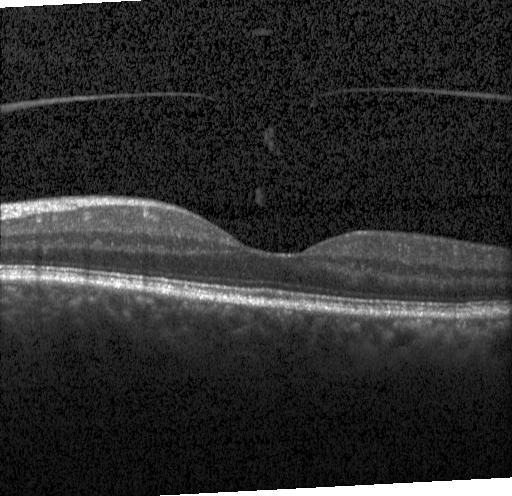 Through the macula. Heidelberg Spectralis. OCT B-scan. Spectral-domain OCT.
No choroidal neovascularization, no diabetic macular edema, and no drusen.